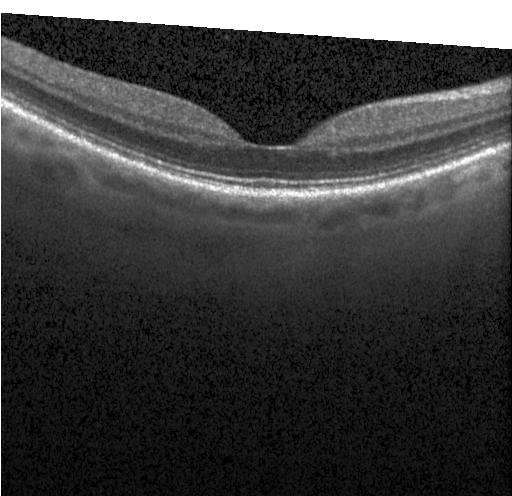

Retinal OCT cross-section.
Impression: no evidence of choroidal neovascularization, diabetic macular edema, or drusen.